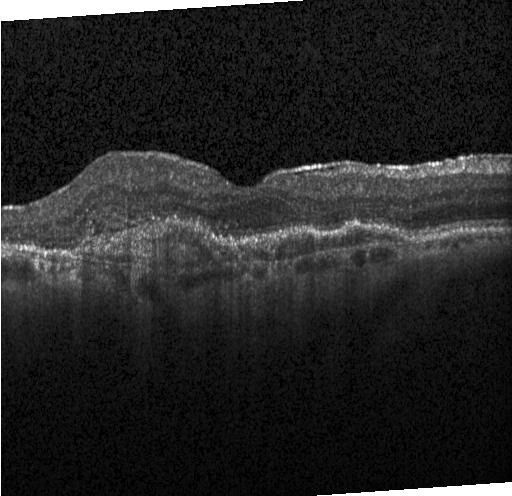 OCT line scan. Finding: a choroidal neovascular membrane.